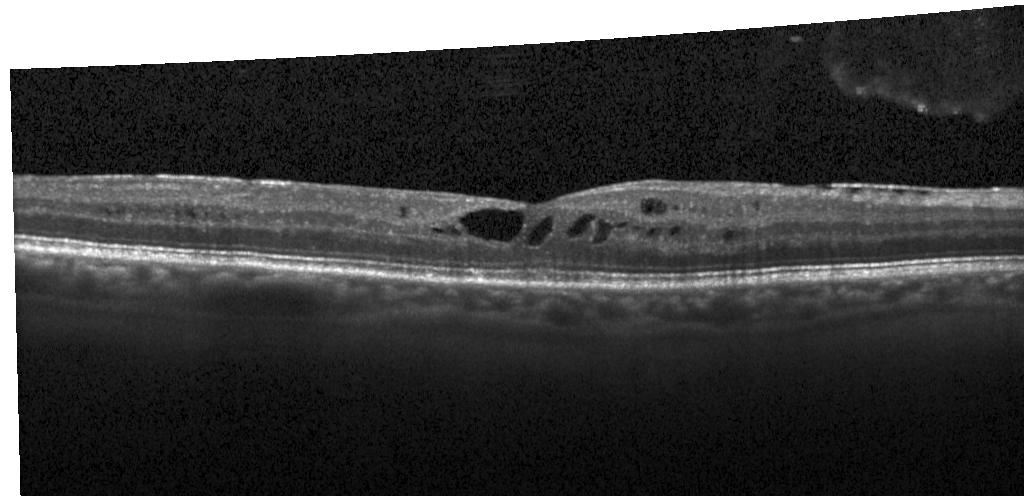
SD-OCT. Centered on the fovea. Heidelberg Spectralis. OCT B-scan
Impression: diabetic macular edema.